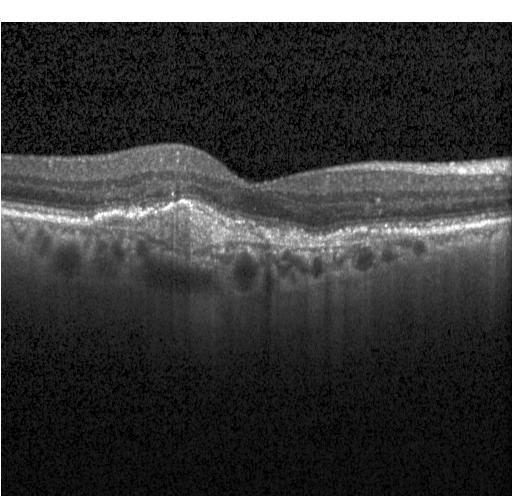
Horizontal scan through the fovea; Heidelberg Spectralis OCT system; OCT line scan; SD-OCT — Assessment: CNV.